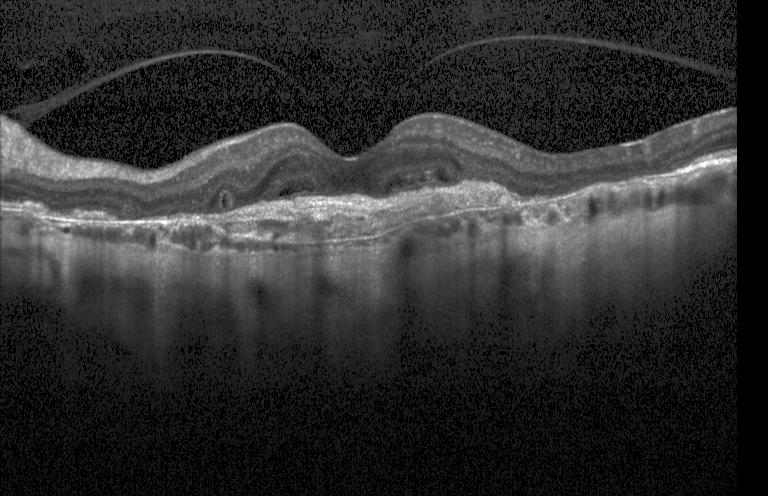

Macular scan. Spectral-domain OCT. Heidelberg Spectralis OCT system. Optical coherence tomography scan.
A choroidal neovascular membrane.